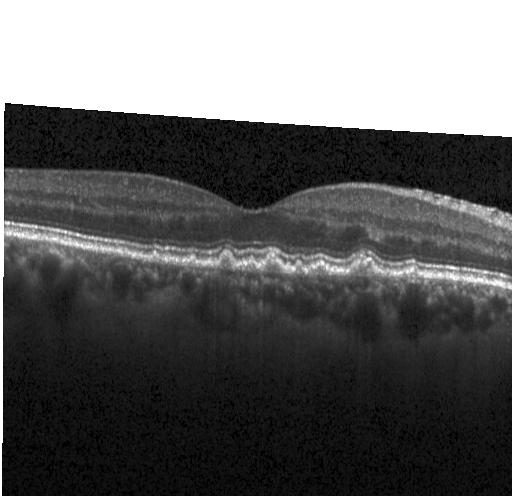 Retinal OCT cross-section — Impression: drusen.